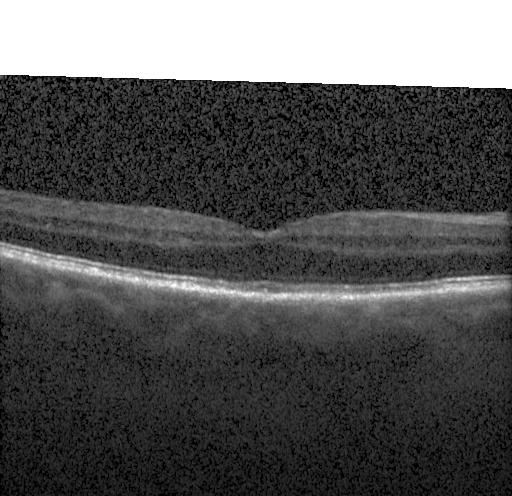

Dx: neither choroidal neovascularization, diabetic macular edema, nor drusen.